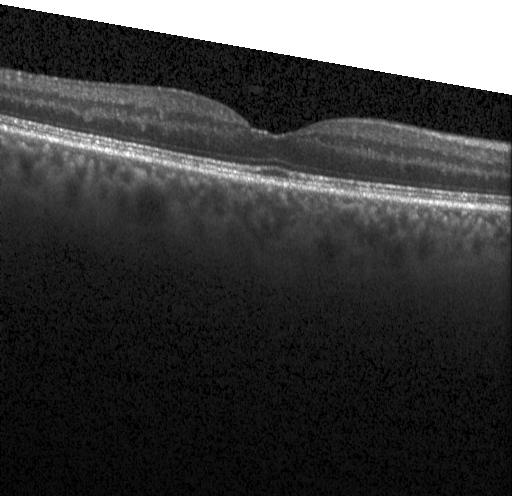
Centered on the fovea · retinal OCT cross-section · instrument: Heidelberg Spectralis — No evidence of choroidal neovascularization, diabetic macular edema, or drusen.